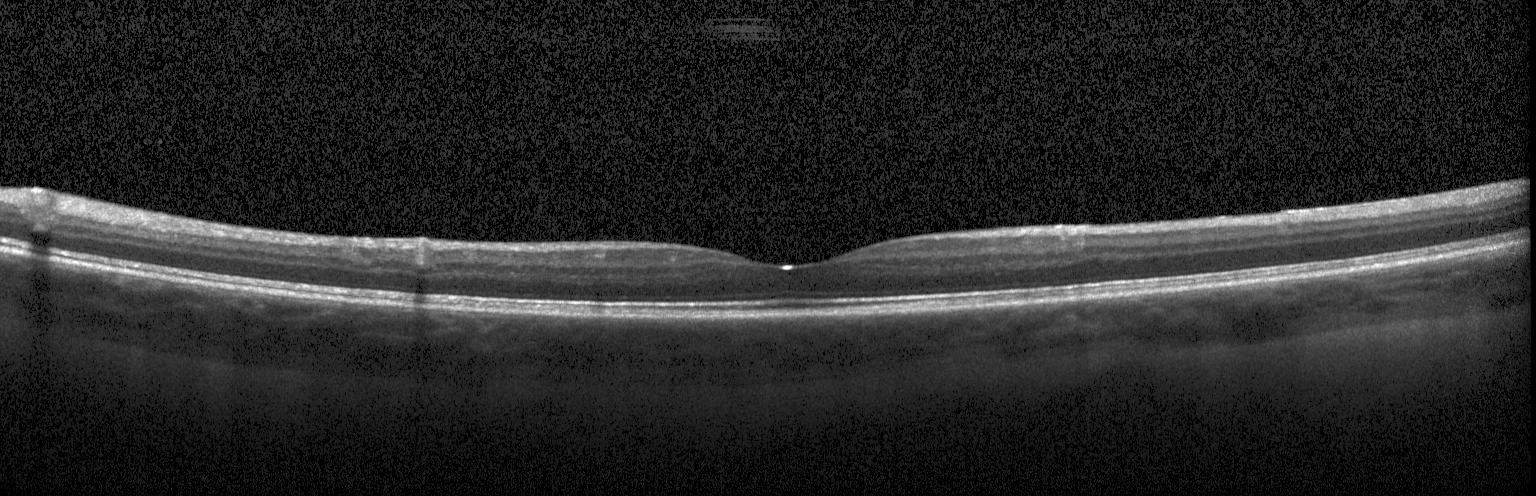 Optical coherence tomography B-scan; acquired on a Heidelberg Spectralis; through the macula.
Finding: no evidence of CNV, DME, or drusen.